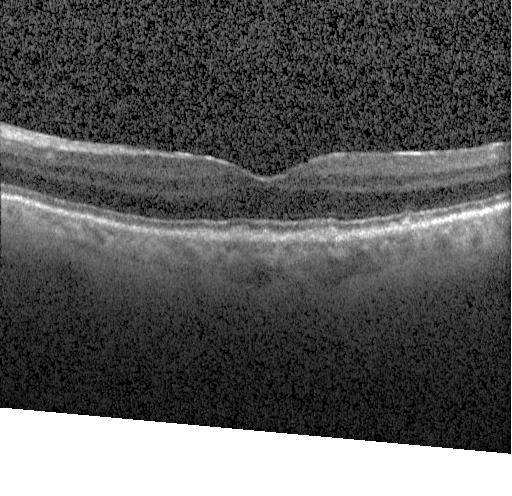 OCT B-scan. Fovea-centered
Multiple drusen.